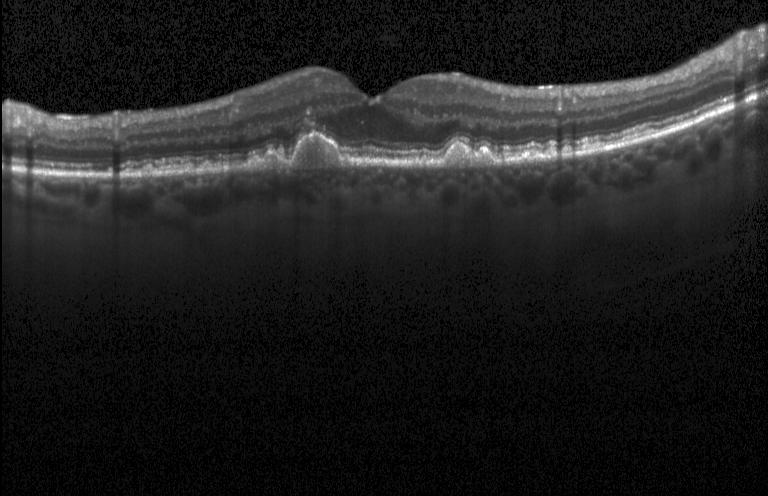 OCT finding: drusen.